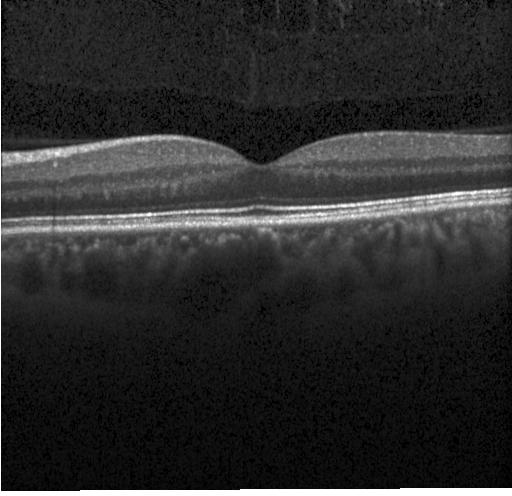

Heidelberg Spectralis OCT system, optical coherence tomography scan.
Diagnosis: no choroidal neovascularization, no diabetic macular edema, and no drusen.